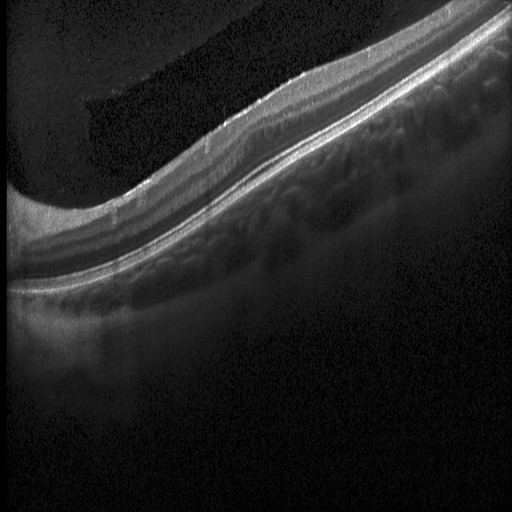

OCT B-scan; SD-OCT.
Macular OCT: diabetic macular edema.